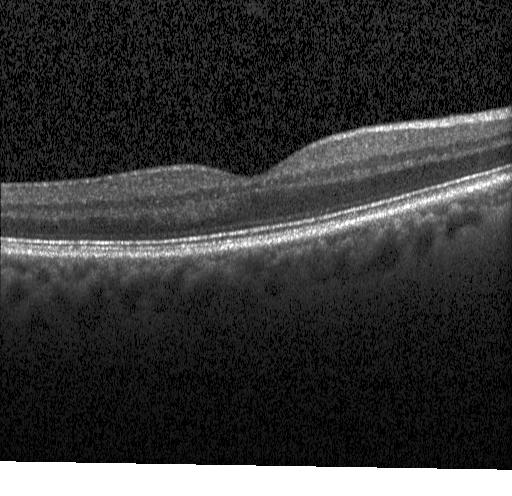 Optical coherence tomography scan.
Finding: no choroidal neovascularization, no diabetic macular edema, and no drusen.